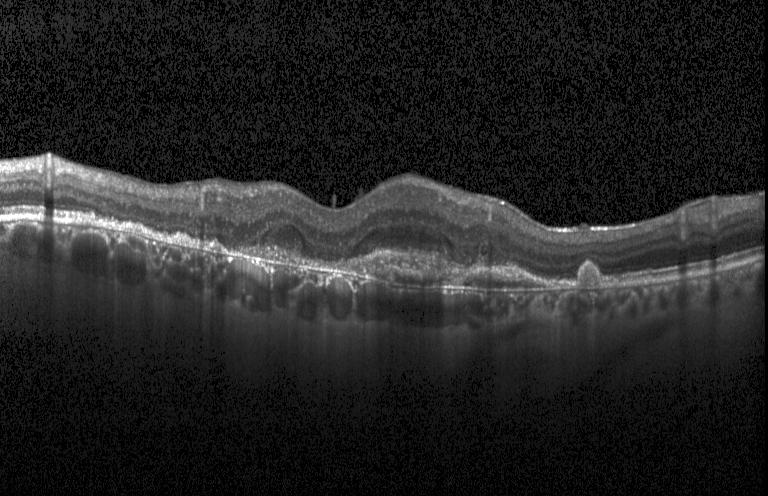 SD-OCT. OCT line scan. Instrument: Heidelberg Spectralis. Fovea-centered
Dx: a choroidal neovascular membrane.